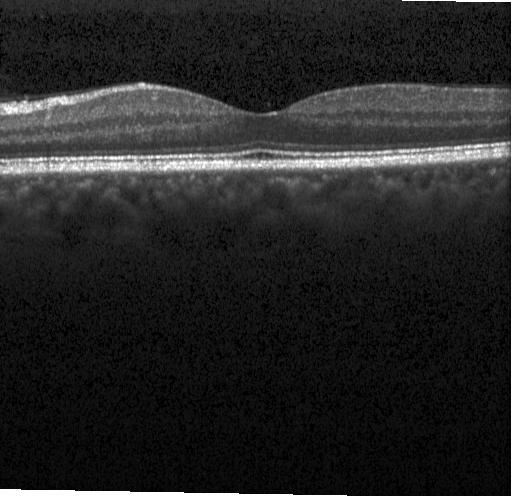
Spectral-domain OCT; retinal OCT B-scan; acquired on a Heidelberg Spectralis
This B-scan demonstrates no CNV, no DME, and no drusen.